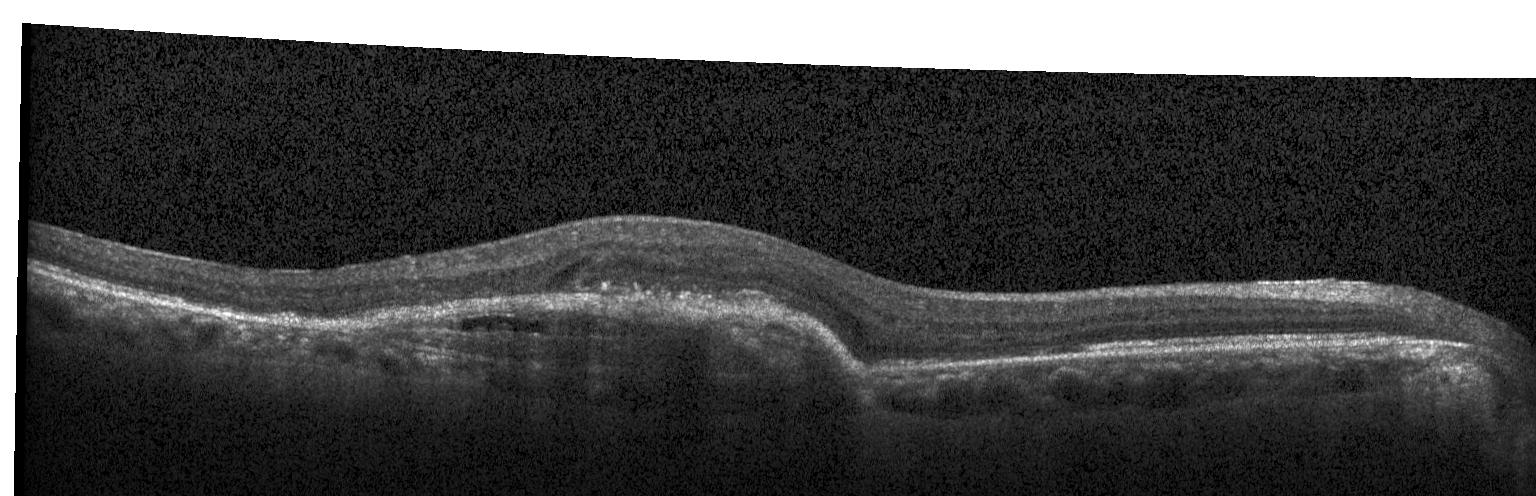
SD-OCT. Through the macula. Heidelberg Spectralis OCT system. Retinal OCT B-scan. The scan shows a choroidal neovascular membrane.